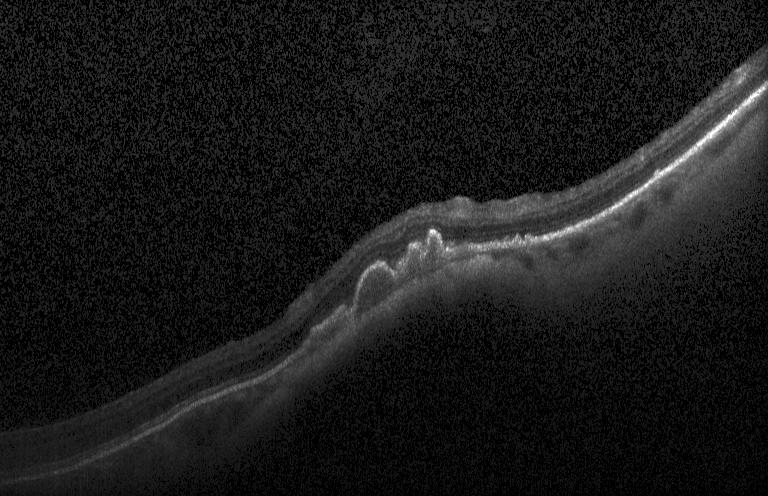
OCT B-scan; fovea-centered.
Macular OCT: CNV.